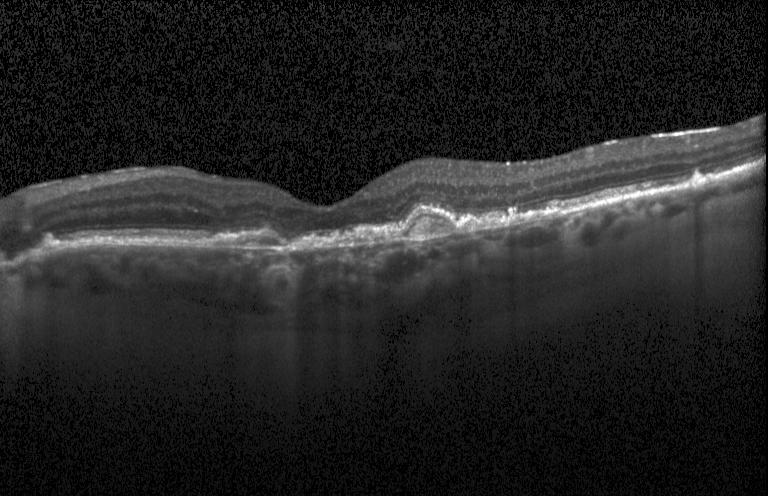
Optical coherence tomography scan, Heidelberg Spectralis, macular scan, SD-OCT.
Diagnosis: a choroidal neovascular membrane.